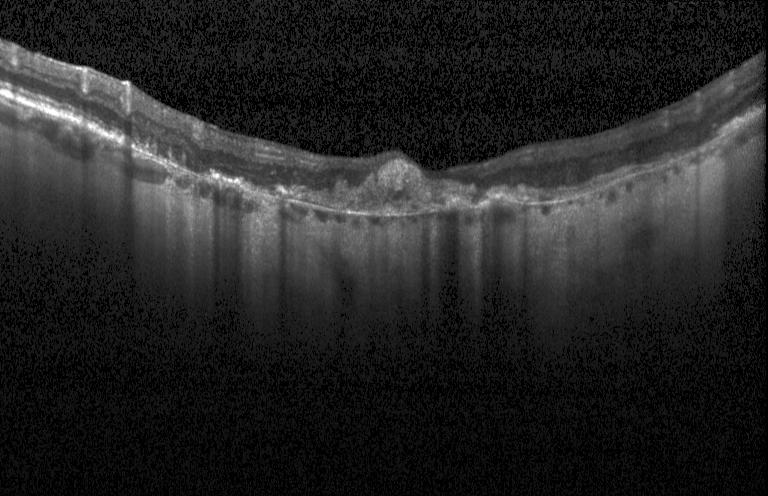 OCT finding: a choroidal neovascular membrane.